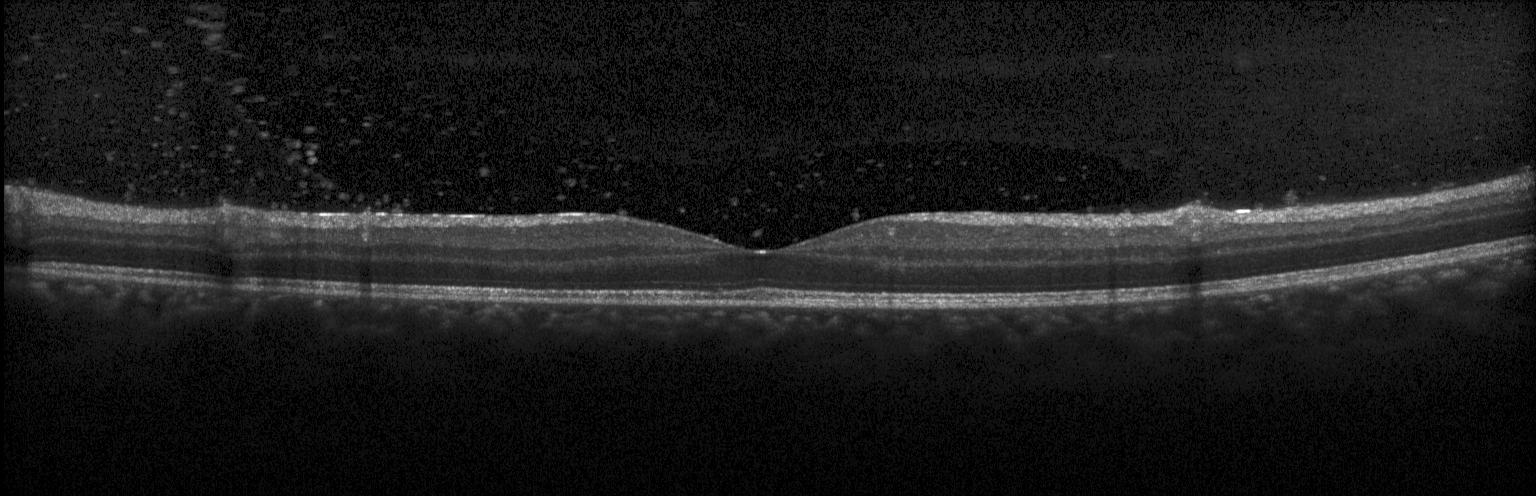

No CNV, no DME, and no drusen.